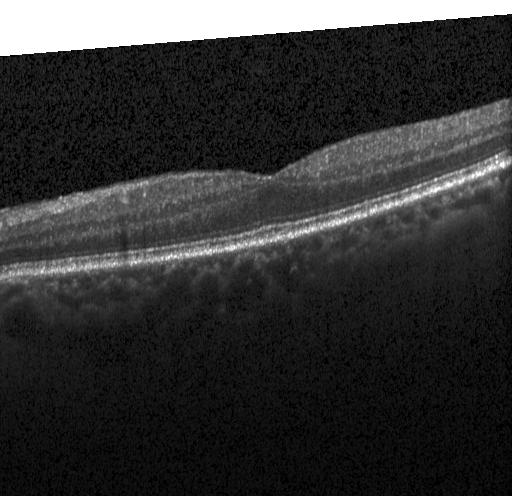 Retinal OCT cross-section.
Finding: neither choroidal neovascularization, diabetic macular edema, nor drusen.